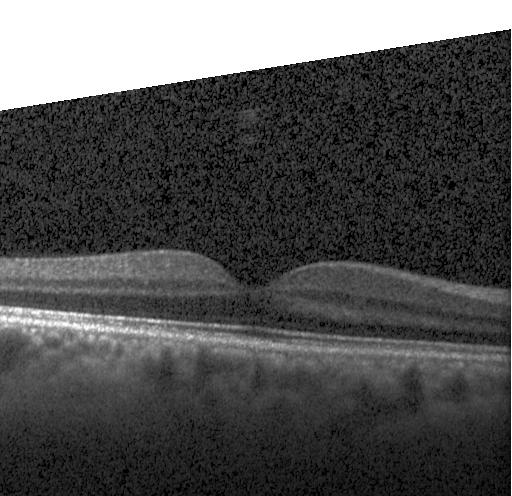 Spectral-domain optical coherence tomography, macular scan, OCT B-scan
Impression: neither choroidal neovascularization, diabetic macular edema, nor drusen.